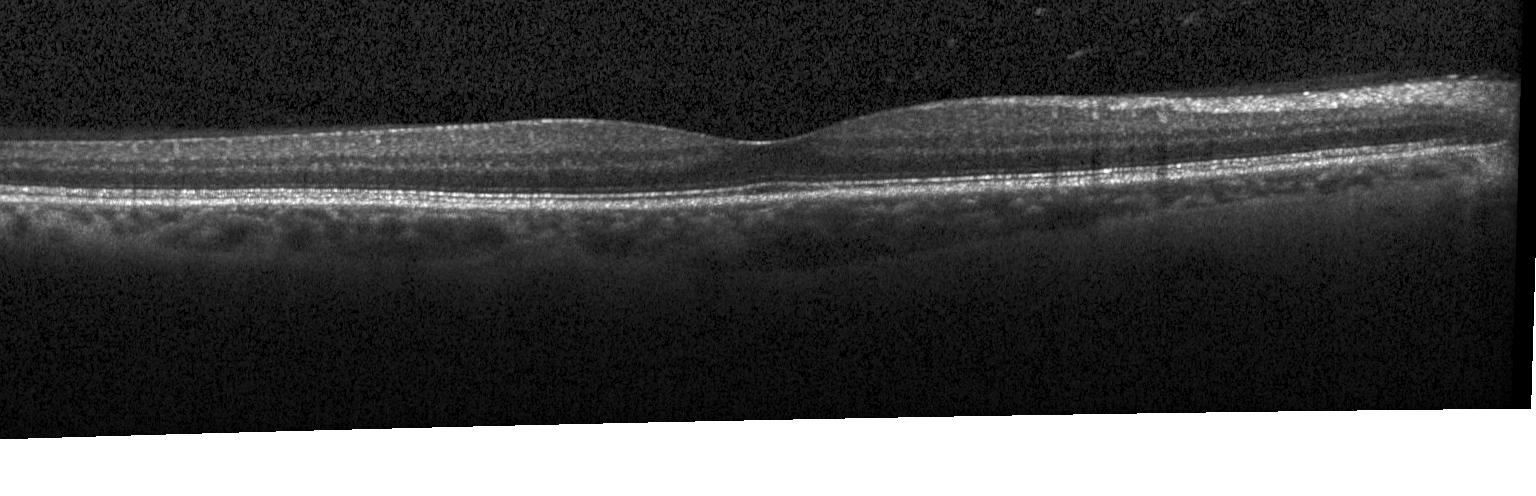
Optical coherence tomography B-scan; fovea-centered. This B-scan demonstrates no CNV, DME, or drusen.